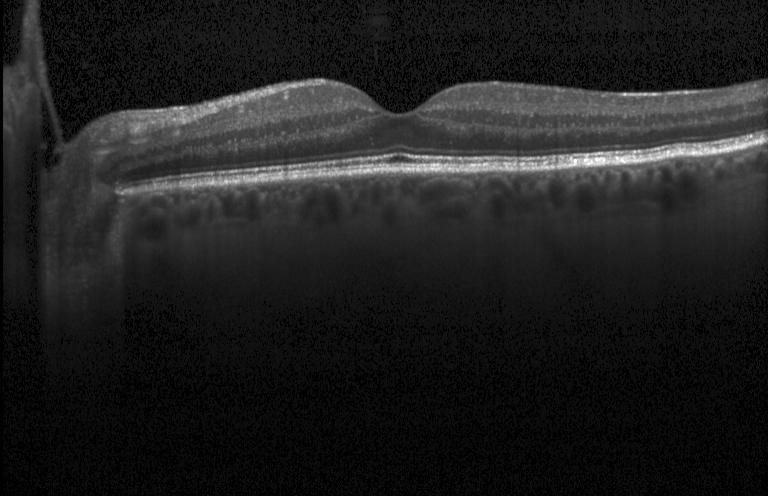 Optical coherence tomography scan
Impression: no CNV, DME, or drusen.